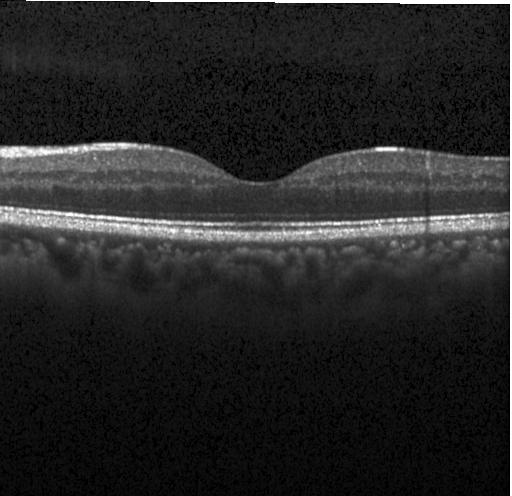

Diagnosis: neither CNV, DME, nor drusen.